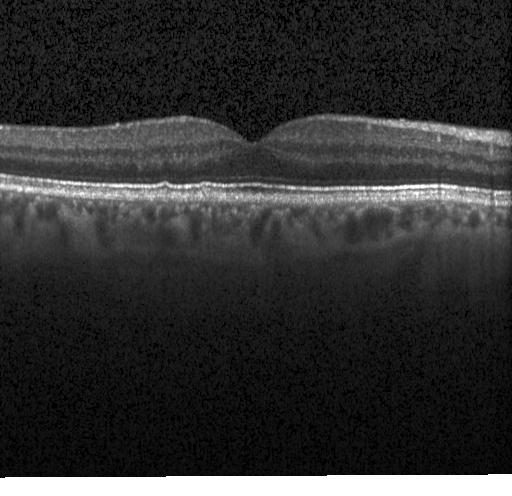

Acquired on a Heidelberg Spectralis. Retinal OCT B-scan — Macular OCT: sub-RPE drusenoid deposits.